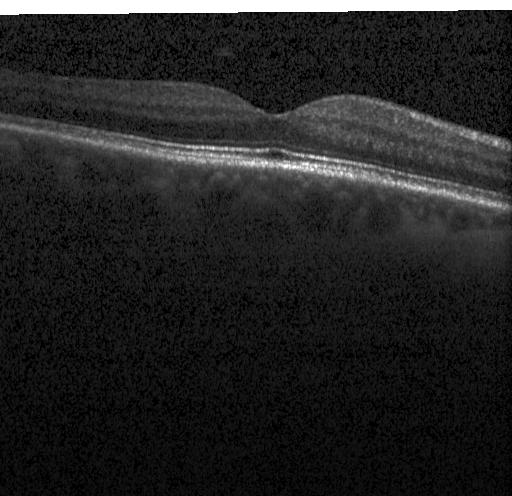
Macular scan. Spectral-domain optical coherence tomography. OCT B-scan
OCT finding: no choroidal neovascularization, diabetic macular edema, or drusen.